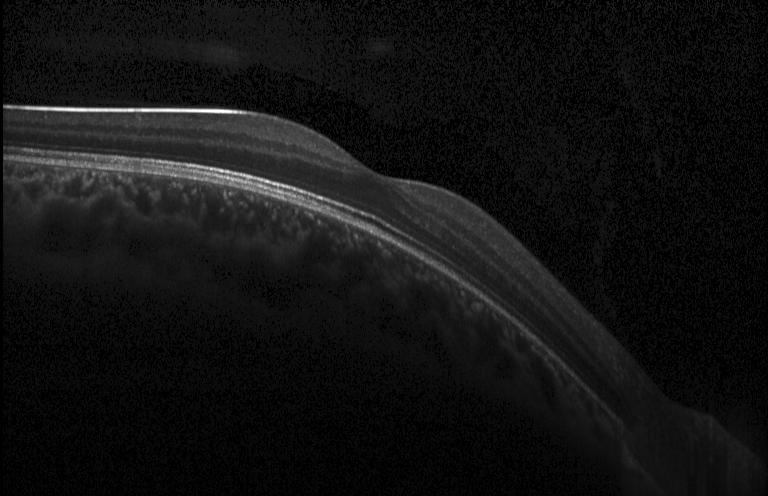 OCT finding: no CNV, DME, or drusen.